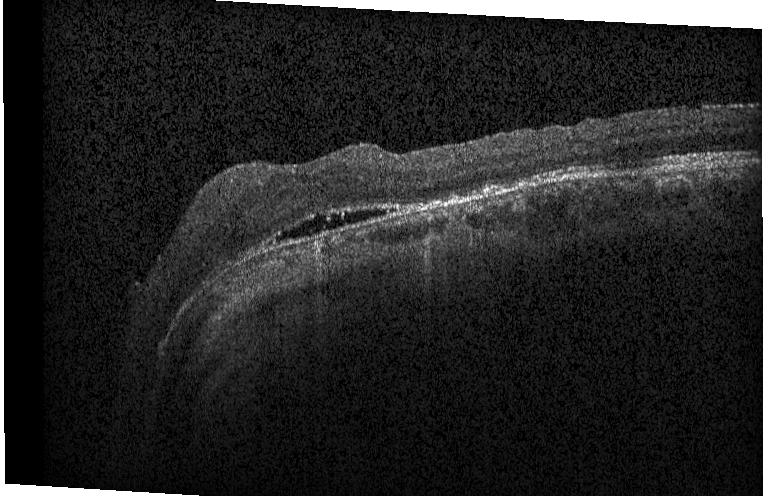
Optical coherence tomography B-scan. Finding: a choroidal neovascular membrane.